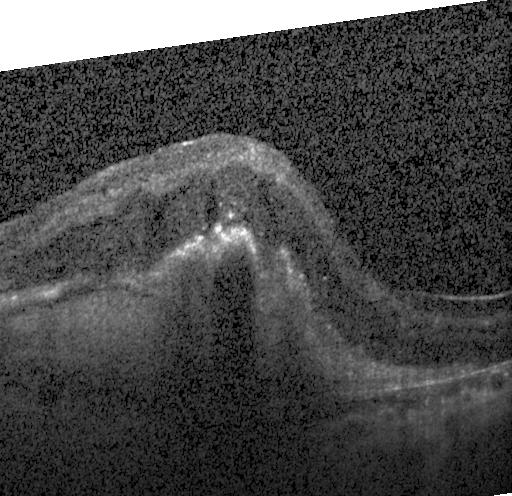 Finding: a choroidal neovascular membrane.